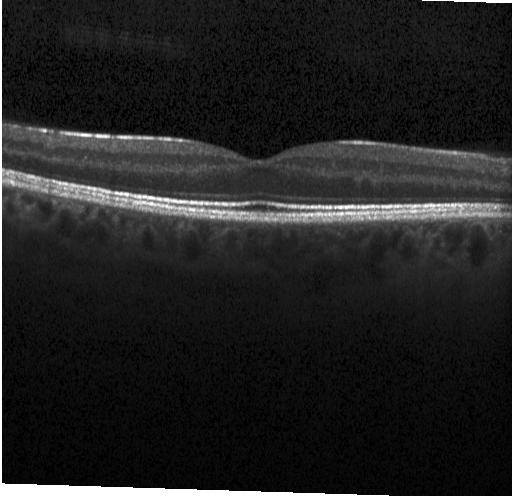

Diagnosis: neither choroidal neovascularization, diabetic macular edema, nor drusen.